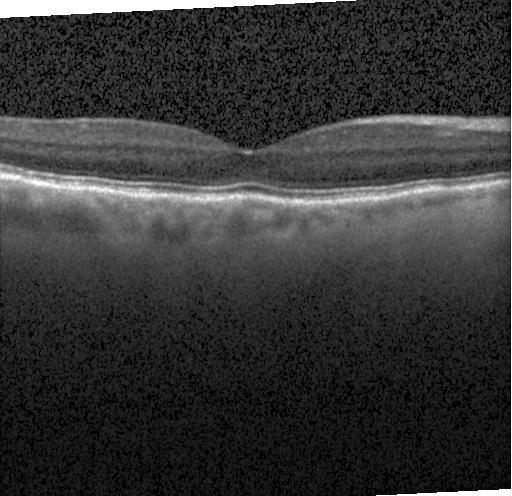 Spectral-domain OCT B-scan: neither choroidal neovascularization, diabetic macular edema, nor drusen.